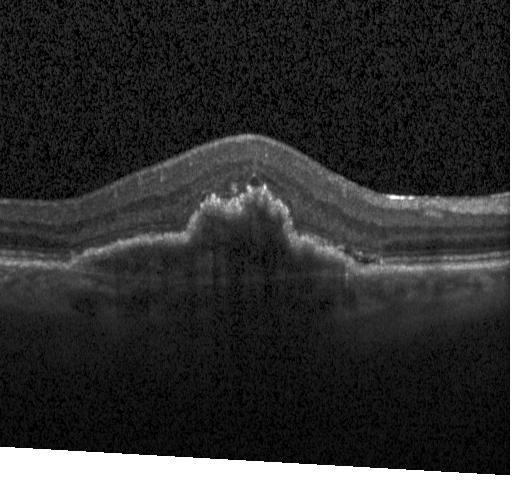 Impression: choroidal neovascularization.